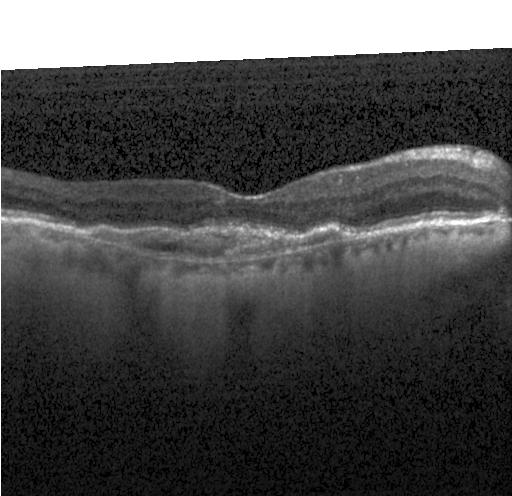 OCT B-scan. Assessment: CNV.